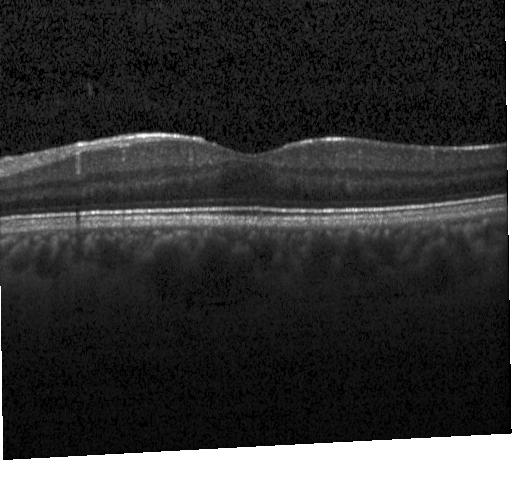
Spectral-domain optical coherence tomography · instrument: Heidelberg Spectralis · retinal OCT B-scan · through the macula.
Diagnosis: no choroidal neovascularization, diabetic macular edema, or drusen.